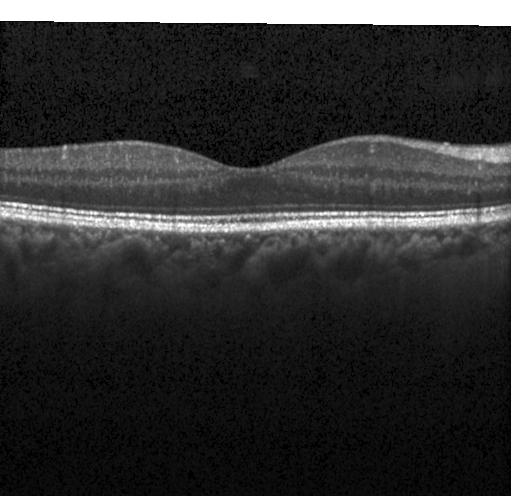

Optical coherence tomography scan.
Impression: no choroidal neovascularization, diabetic macular edema, or drusen.